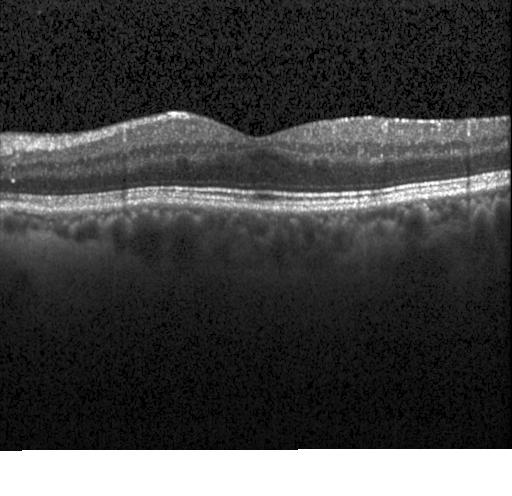

Heidelberg Spectralis OCT system; through the macula; optical coherence tomography B-scan; spectral-domain OCT — Finding: no evidence of CNV, DME, or drusen.